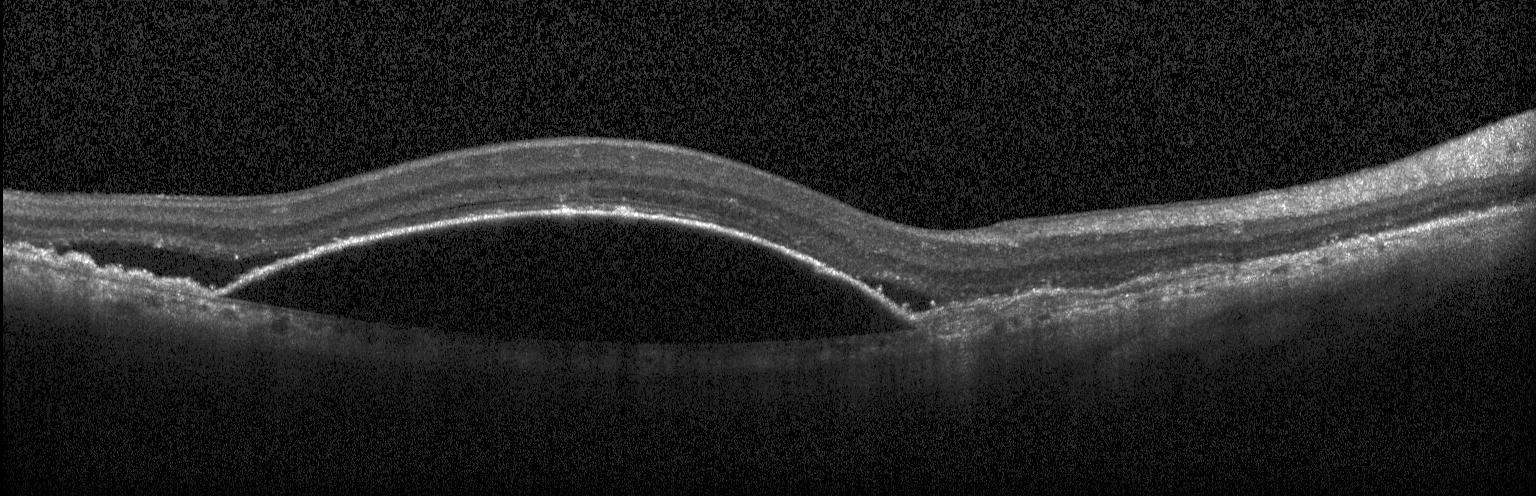 Macular OCT demonstrating a choroidal neovascular membrane.